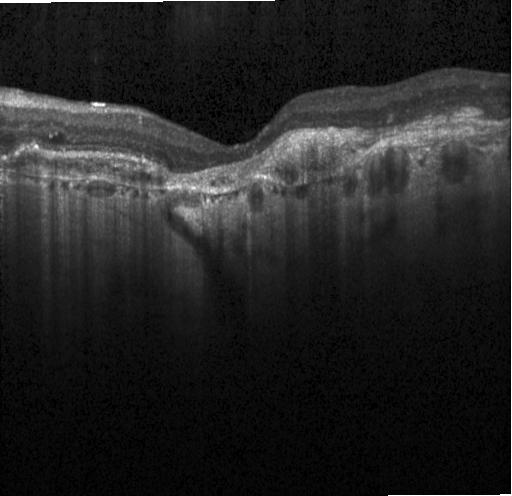

Optical coherence tomography scan. Heidelberg Spectralis. SD-OCT. The scan shows a choroidal neovascular membrane.